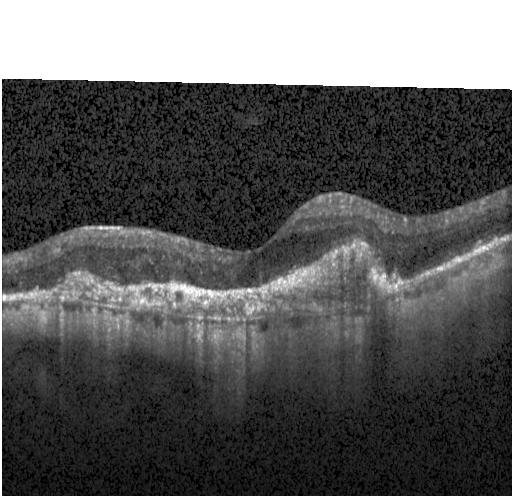 This B-scan demonstrates choroidal neovascularization (CNV).